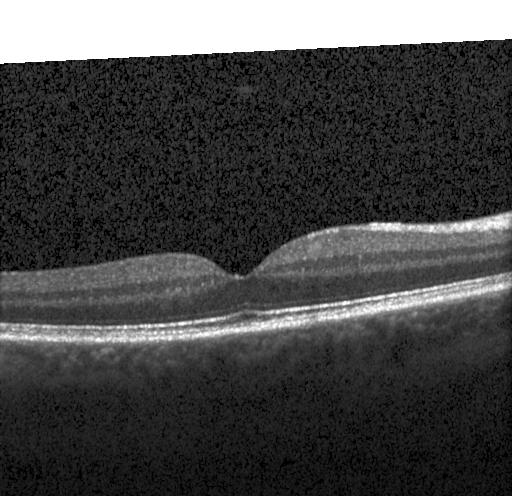
SD-OCT · retinal OCT B-scan.
Diagnosis: no evidence of choroidal neovascularization, diabetic macular edema, or drusen.